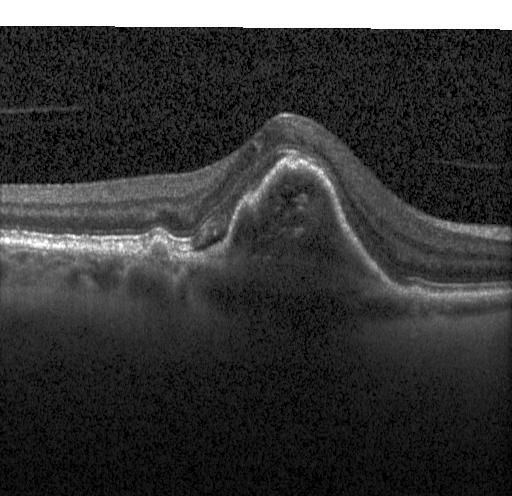

OCT line scan, through the macula, spectral-domain OCT — Dx: a choroidal neovascular membrane.